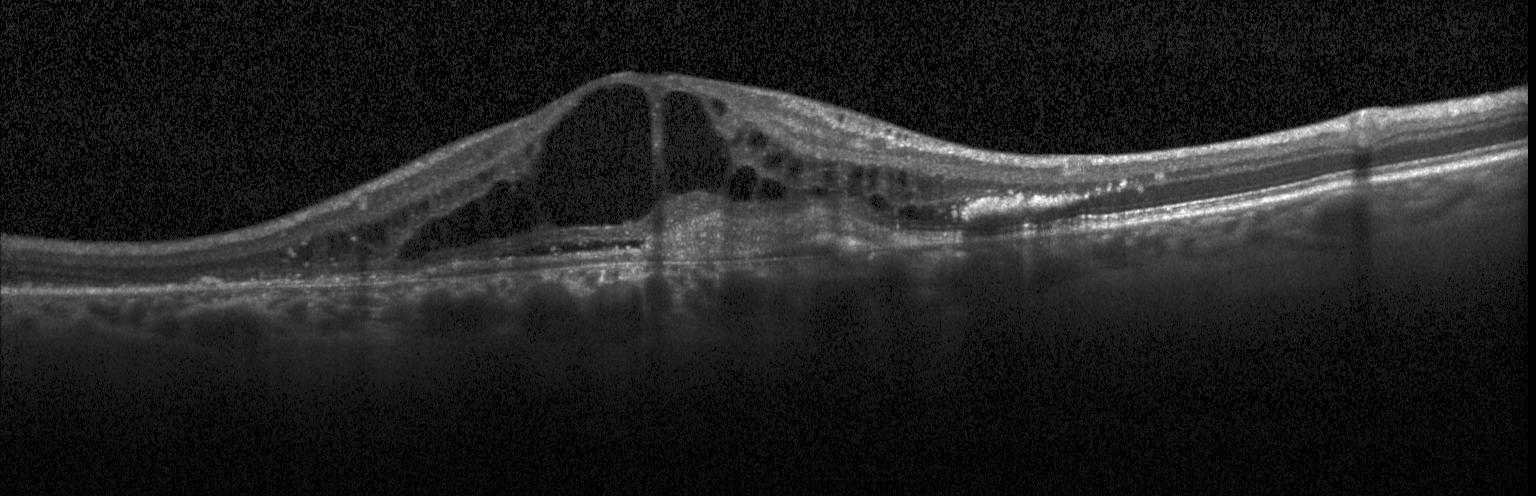
Macular OCT: a choroidal neovascular membrane.